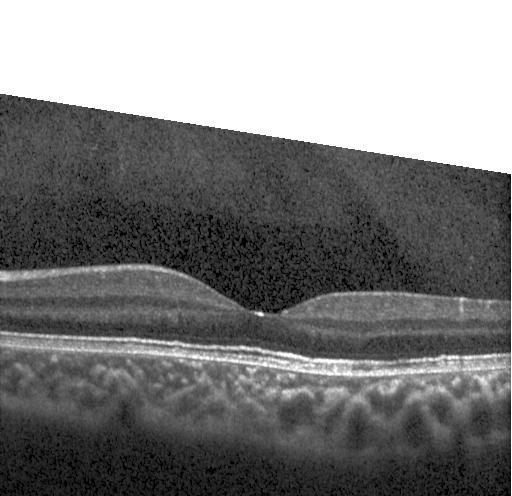

Retinal OCT cross-section · through the macula · SD-OCT — The scan shows no evidence of choroidal neovascularization, diabetic macular edema, or drusen.